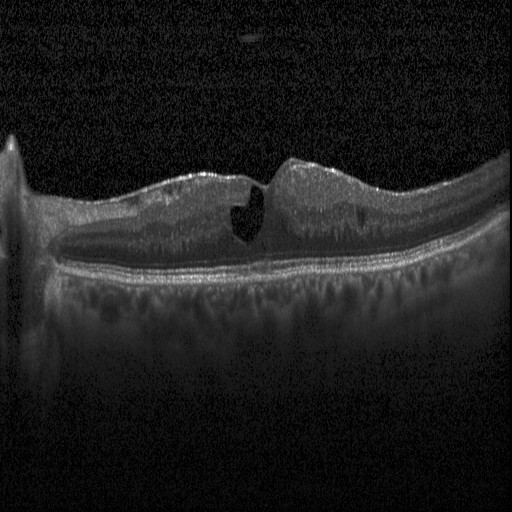 Optical coherence tomography B-scan.
OCT finding: diabetic macular edema.